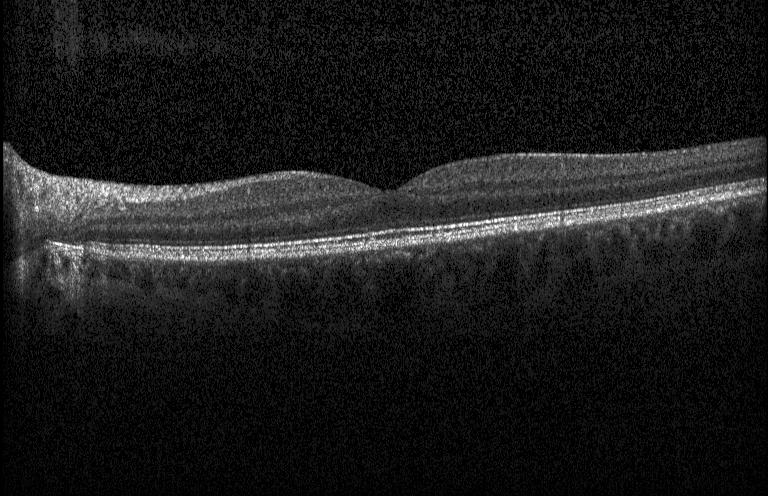

Optical coherence tomography B-scan. Diagnosis: no CNV, no DME, and no drusen.